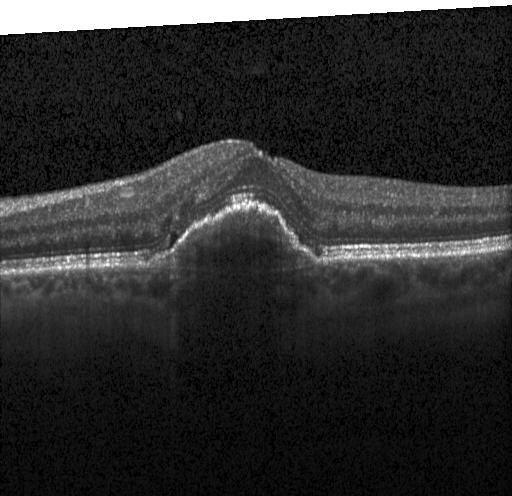 A choroidal neovascular membrane.